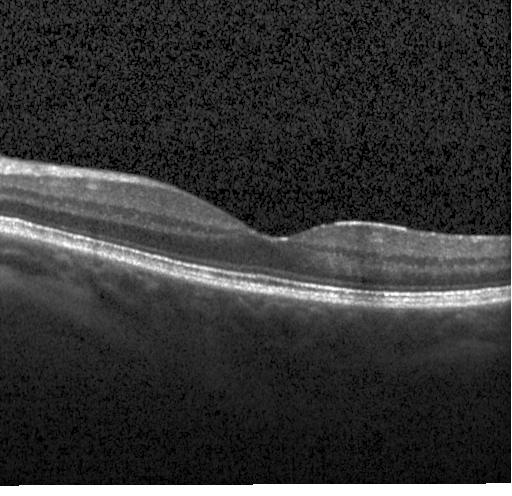 OCT scan showing no CNV, DME, or drusen.